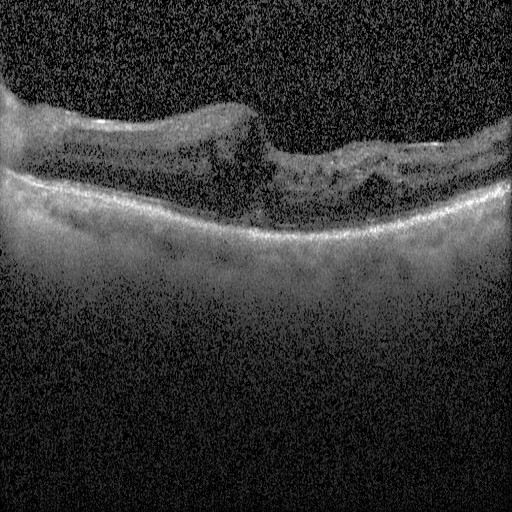 Assessment: DME.